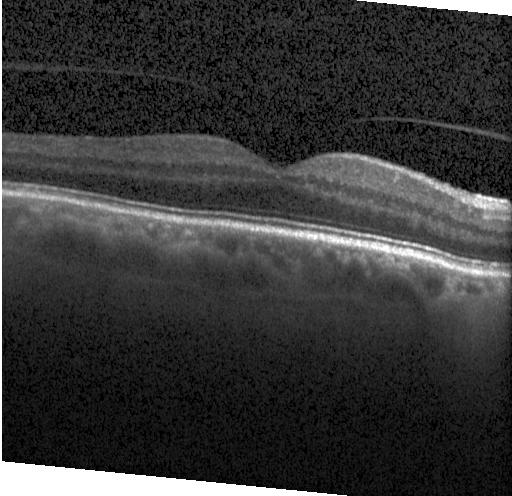 Horizontal scan through the fovea. Retinal OCT B-scan. Finding: no evidence of choroidal neovascularization, diabetic macular edema, or drusen.